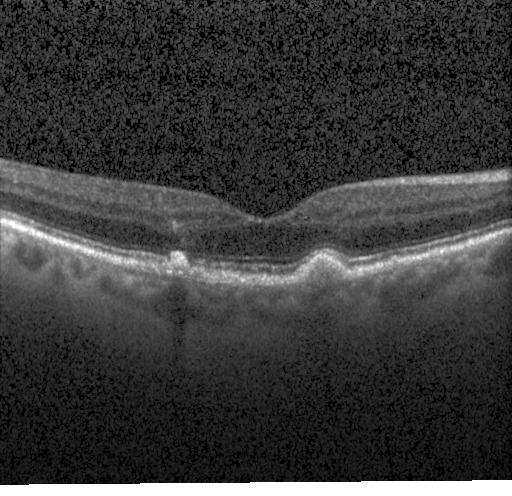
Spectral-domain optical coherence tomography. Instrument: Heidelberg Spectralis. Horizontal scan through the fovea. OCT line scan — Drusen.